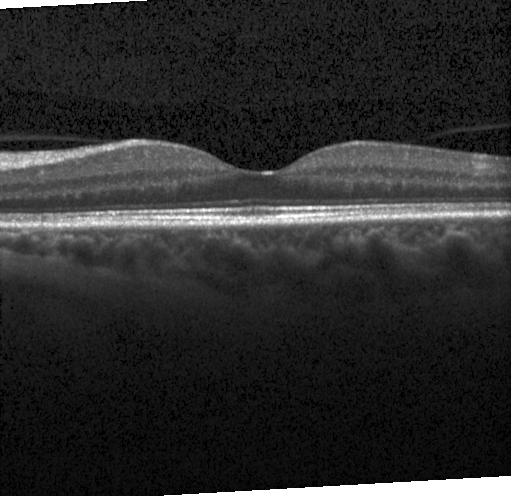

Optical coherence tomography scan · through the macula · Heidelberg Spectralis · spectral-domain optical coherence tomography. Neither choroidal neovascularization, diabetic macular edema, nor drusen.